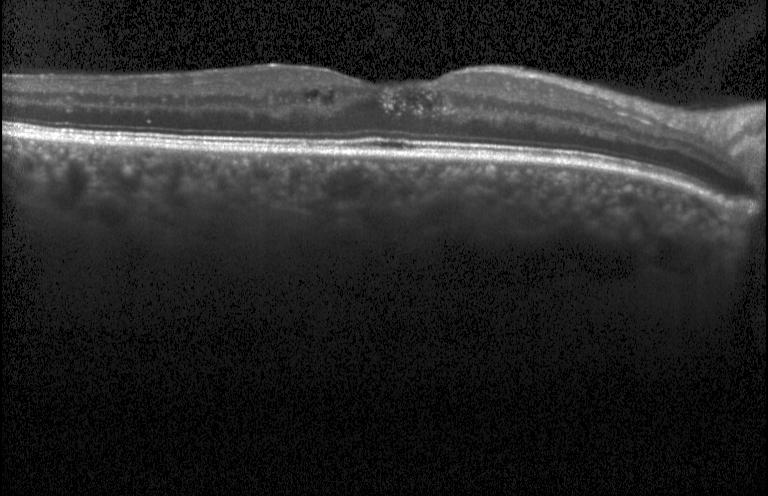 Assessment: DME.